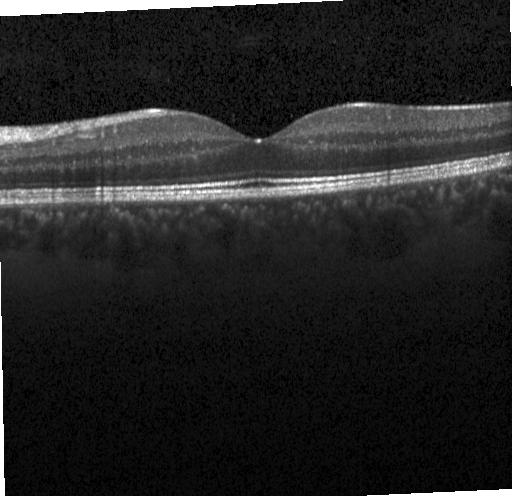
Centered on the fovea. Heidelberg Spectralis OCT system. OCT line scan
Finding: neither choroidal neovascularization, diabetic macular edema, nor drusen.